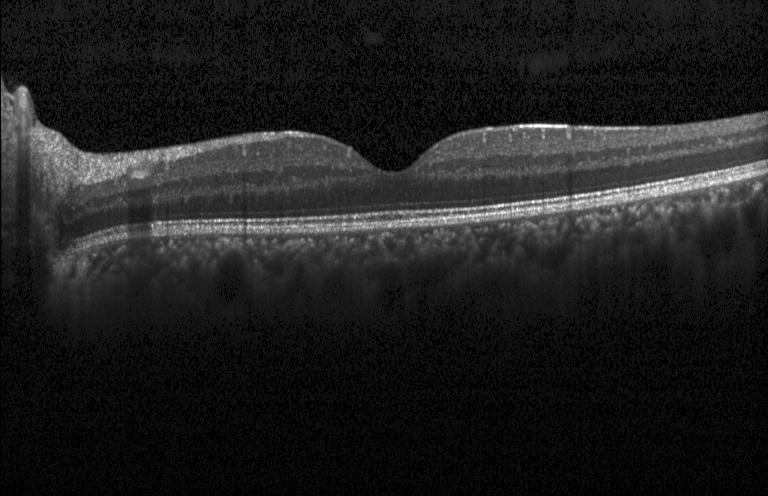

SD-OCT, optical coherence tomography B-scan
Macular OCT: no choroidal neovascularization, diabetic macular edema, or drusen.